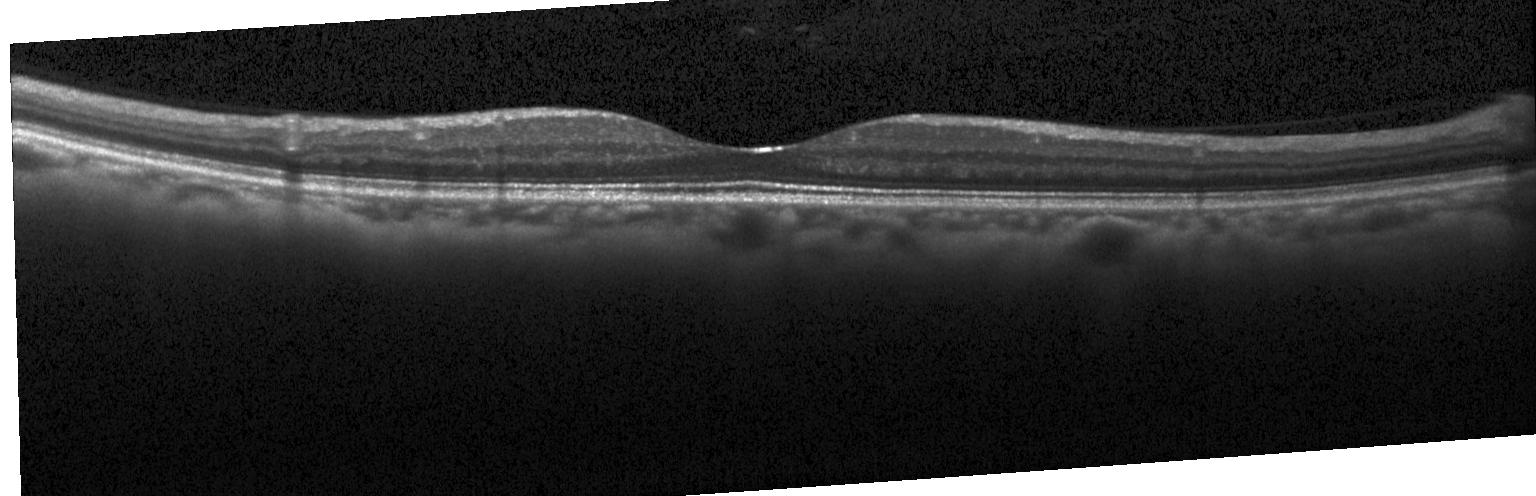
Horizontal scan through the fovea. Heidelberg Spectralis OCT system. Retinal OCT B-scan. Neither choroidal neovascularization, diabetic macular edema, nor drusen.